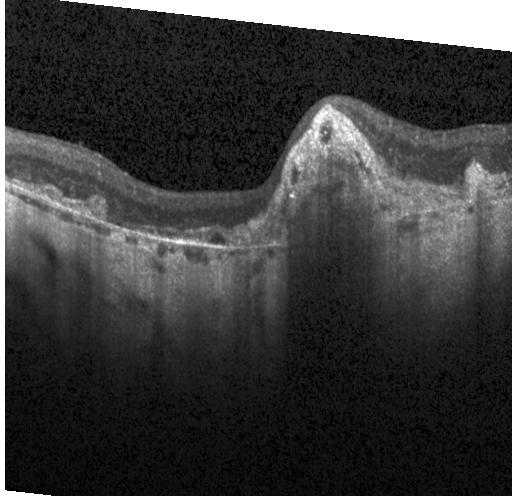 Optical coherence tomography B-scan — Diagnosis: a choroidal neovascular membrane.